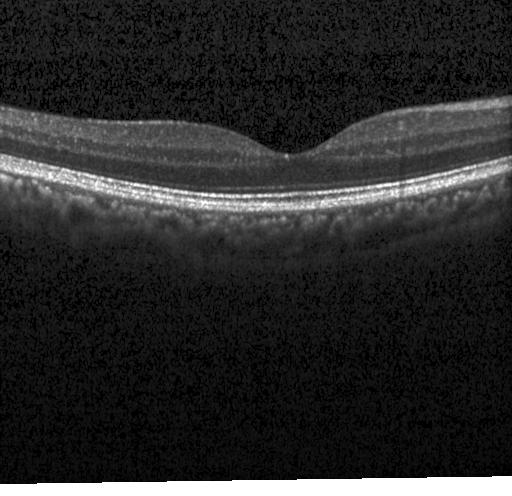
Impression: no choroidal neovascularization, diabetic macular edema, or drusen.